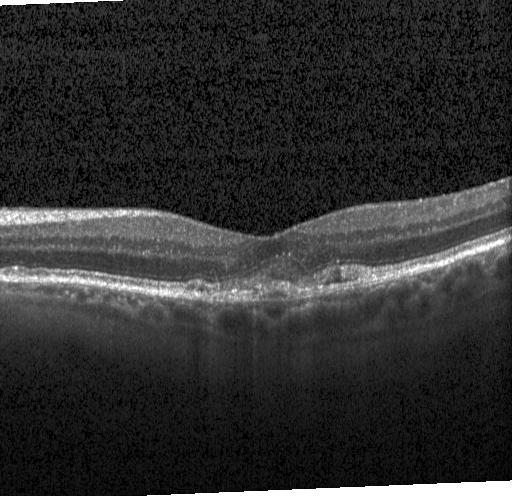 Spectral-domain optical coherence tomography, instrument: Heidelberg Spectralis, macular scan, retinal OCT cross-section.
Macular OCT: CNV.